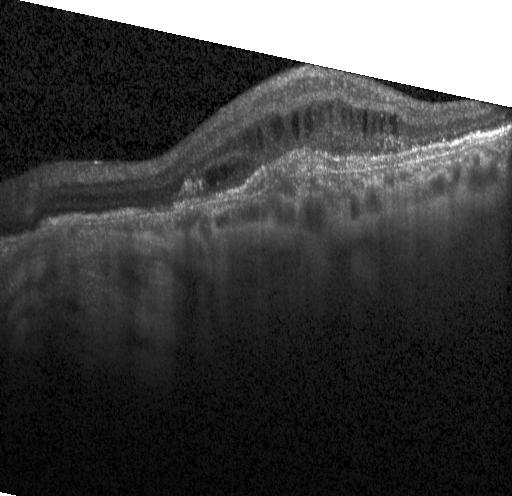

Spectral-domain optical coherence tomography · centered on the fovea · optical coherence tomography B-scan
This B-scan demonstrates choroidal neovascularization.